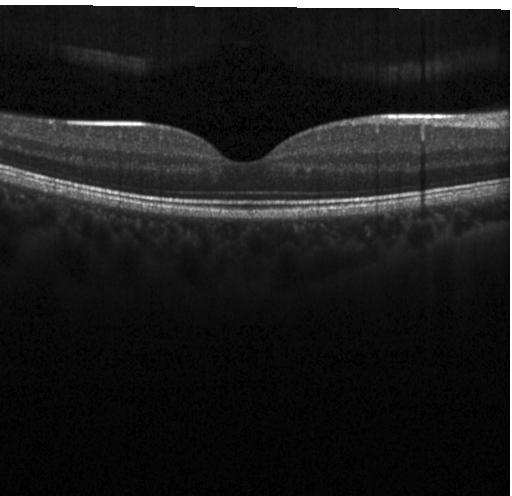
Spectral-domain OCT · OCT line scan · macular scan
No evidence of choroidal neovascularization, diabetic macular edema, or drusen.